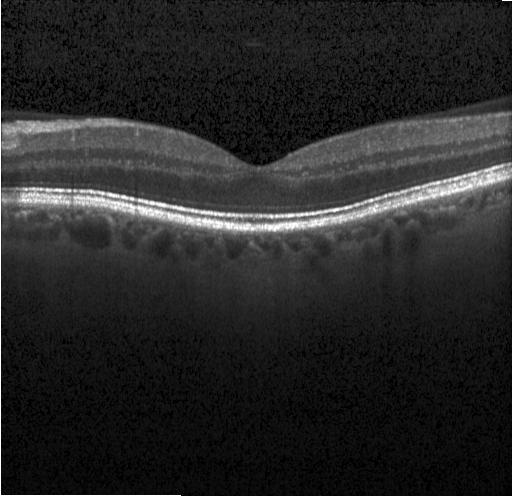 Horizontal scan through the fovea · optical coherence tomography B-scan · acquired on a Heidelberg Spectralis.
No evidence of CNV, DME, or drusen.